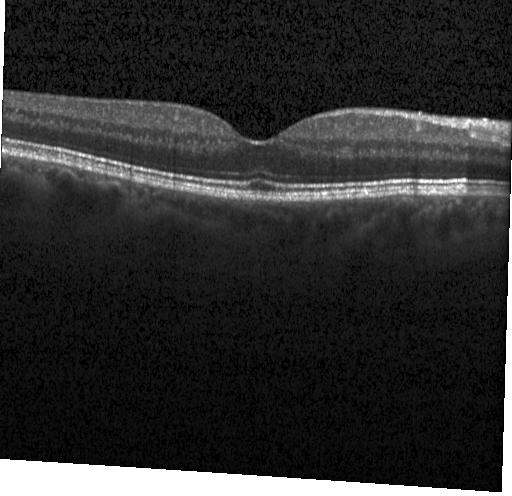

Heidelberg Spectralis OCT system · optical coherence tomography B-scan · SD-OCT. Impression: no choroidal neovascularization, diabetic macular edema, or drusen.